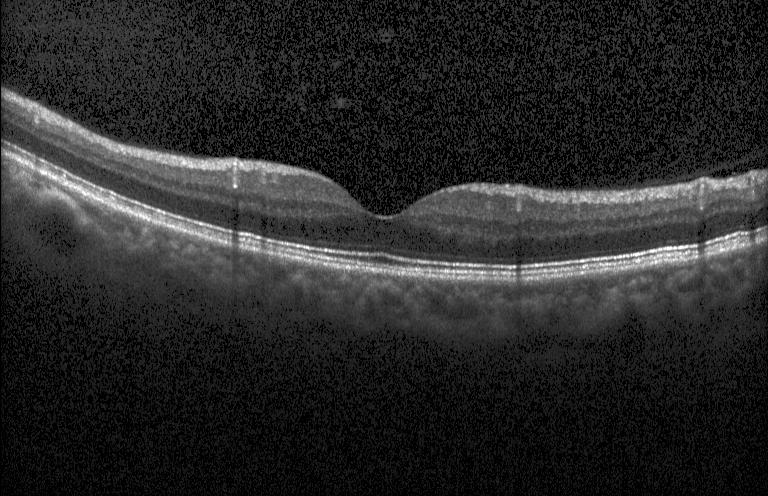 The scan shows no evidence of choroidal neovascularization, diabetic macular edema, or drusen.